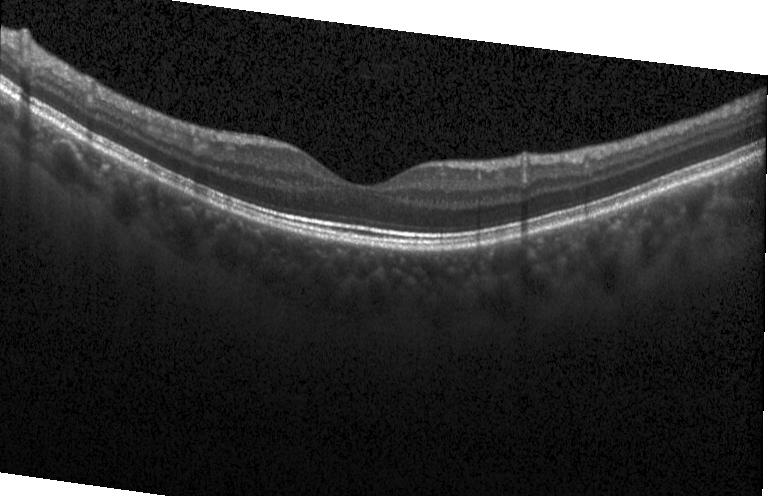
Heidelberg Spectralis · spectral-domain OCT · optical coherence tomography scan · fovea-centered.
Dx: no choroidal neovascularization, diabetic macular edema, or drusen.